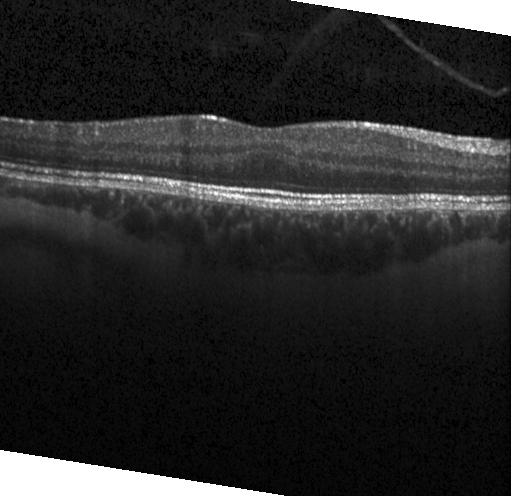

This B-scan demonstrates no evidence of CNV, DME, or drusen.